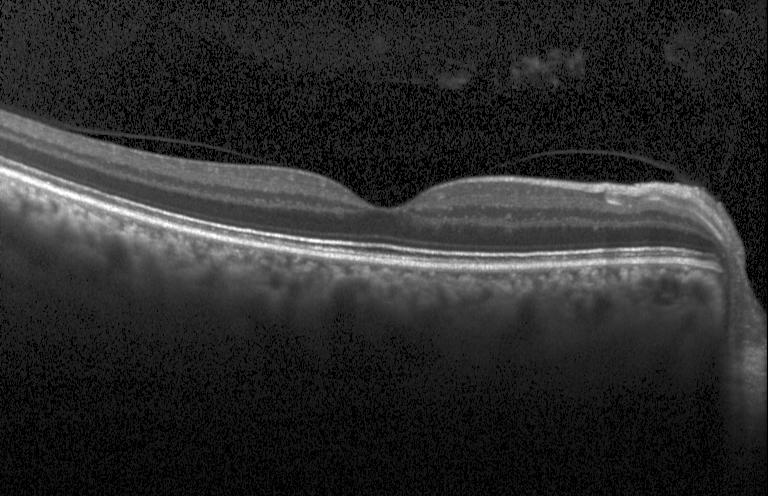

OCT B-scan showing no evidence of CNV, DME, or drusen.